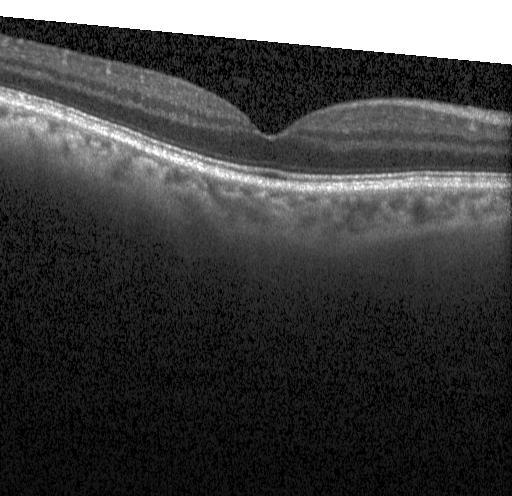
Optical coherence tomography scan · instrument: Heidelberg Spectralis · SD-OCT. The scan shows no CNV, no DME, and no drusen.